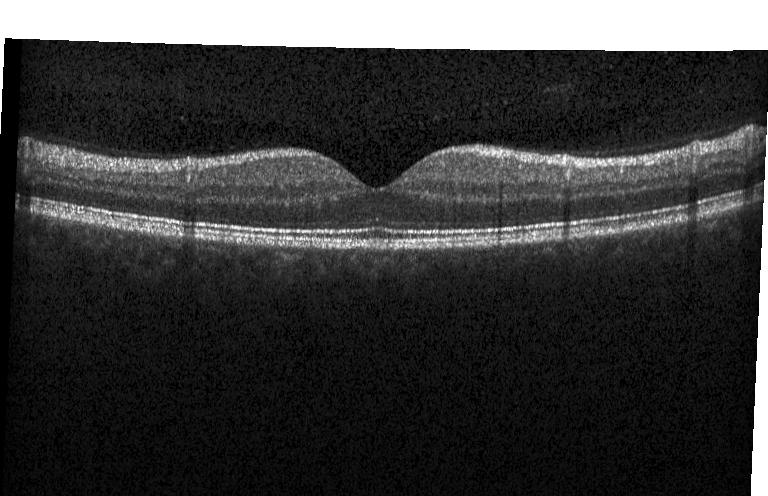
Dx: no CNV, DME, or drusen.